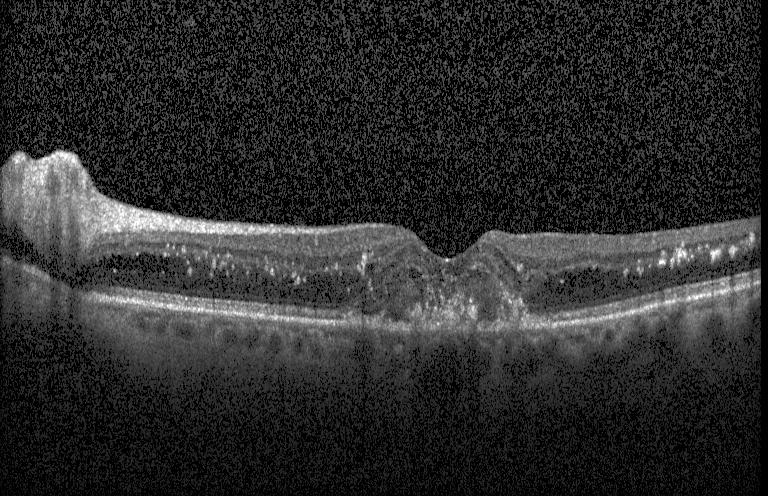

Spectral-domain optical coherence tomography, optical coherence tomography scan — Diagnosis: a choroidal neovascular membrane.